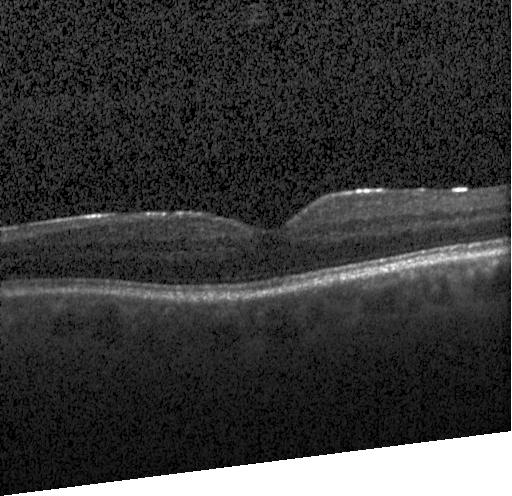

Macular OCT: no choroidal neovascularization, diabetic macular edema, or drusen.